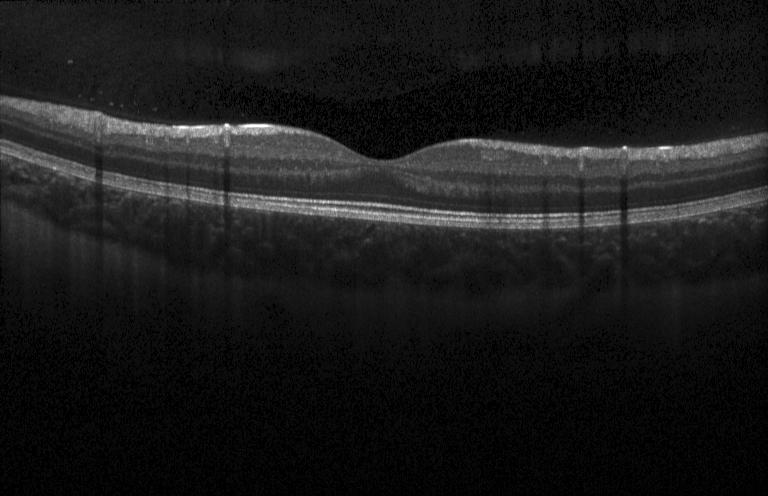 OCT B-scan showing no evidence of choroidal neovascularization, diabetic macular edema, or drusen.